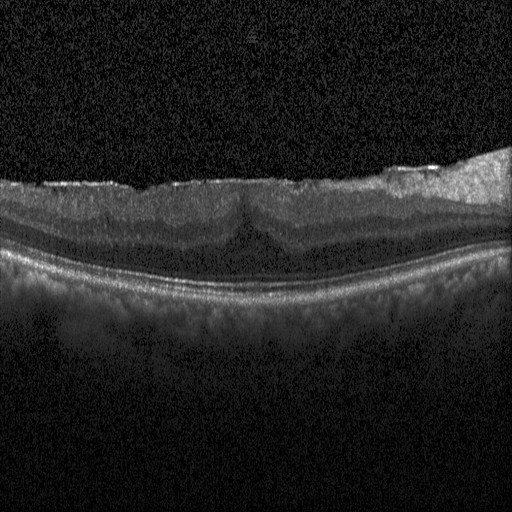 Optical coherence tomography B-scan; Heidelberg Spectralis; macular scan; spectral-domain optical coherence tomography
Diagnosis: diabetic macular edema (DME).